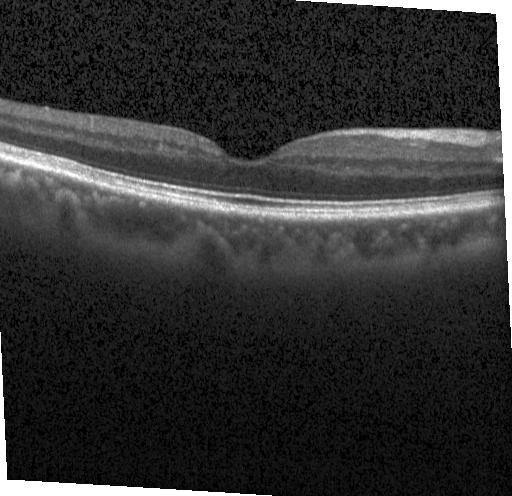 OCT line scan. Heidelberg Spectralis OCT system. Fovea-centered
This B-scan demonstrates no evidence of CNV, DME, or drusen.